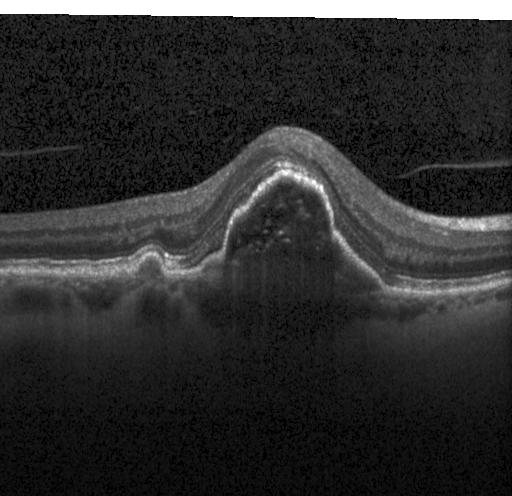

SD-OCT · optical coherence tomography B-scan · Heidelberg Spectralis OCT system · fovea-centered. OCT finding: a choroidal neovascular membrane.